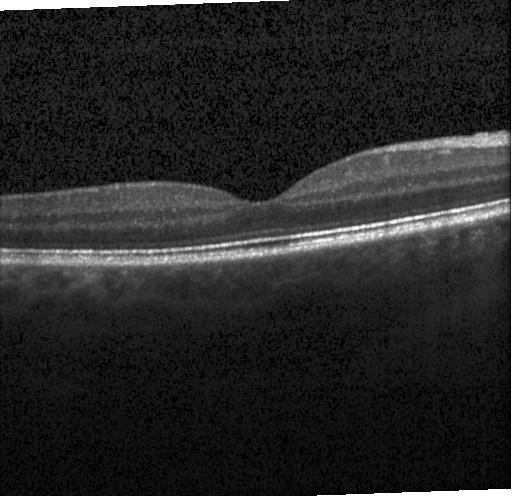
OCT finding: neither choroidal neovascularization, diabetic macular edema, nor drusen.